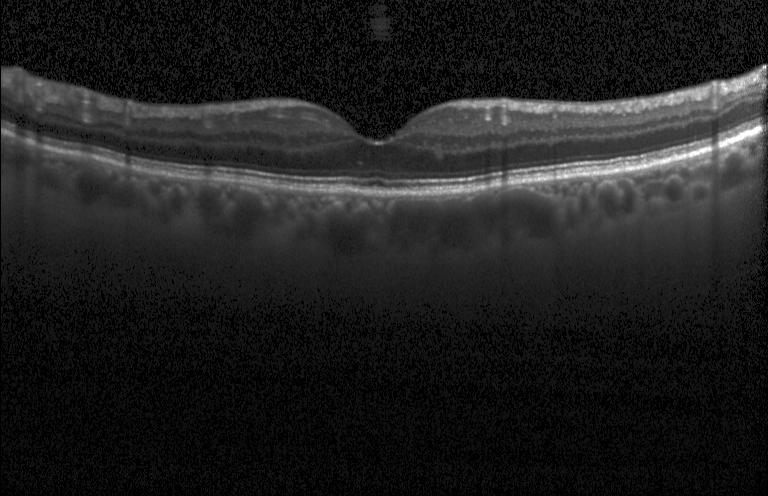 OCT finding: no CNV, no DME, and no drusen.